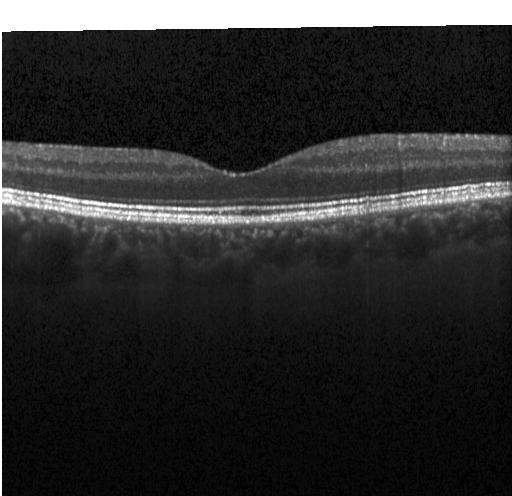
Spectral-domain OCT B-scan: no choroidal neovascularization, diabetic macular edema, or drusen.